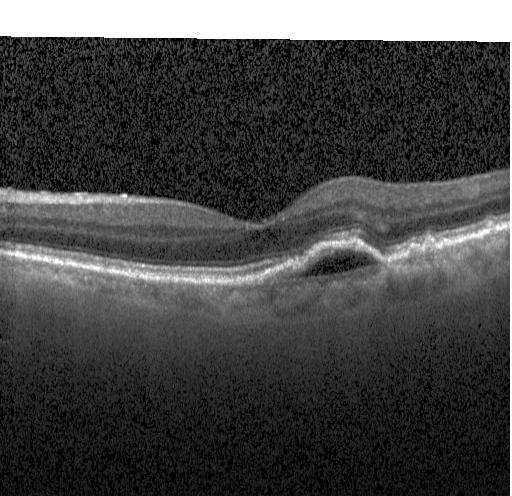
OCT finding: a choroidal neovascular membrane.